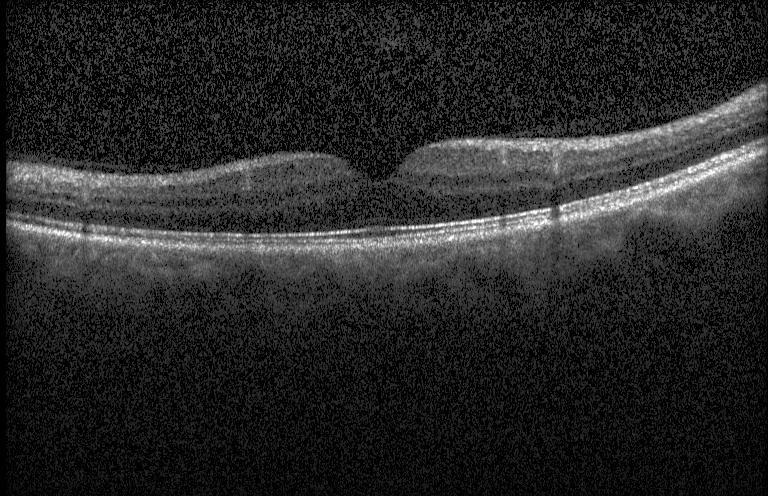
Macular scan, retinal OCT B-scan. OCT finding: no CNV, no DME, and no drusen.